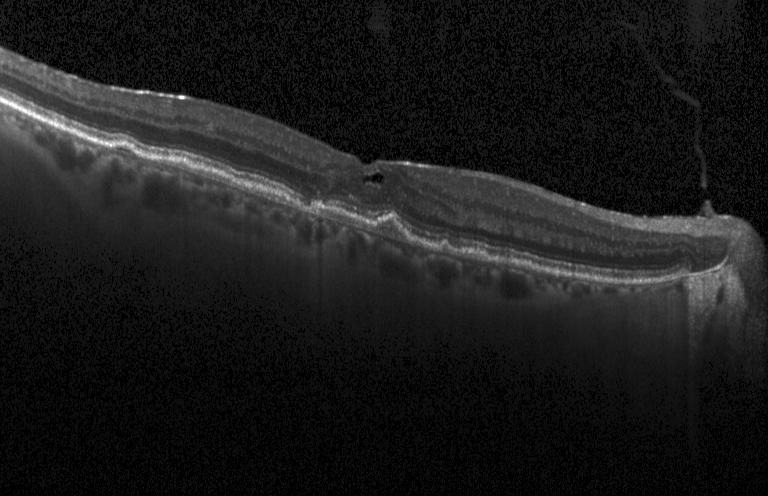

Retinal OCT cross-section showing a choroidal neovascular membrane.